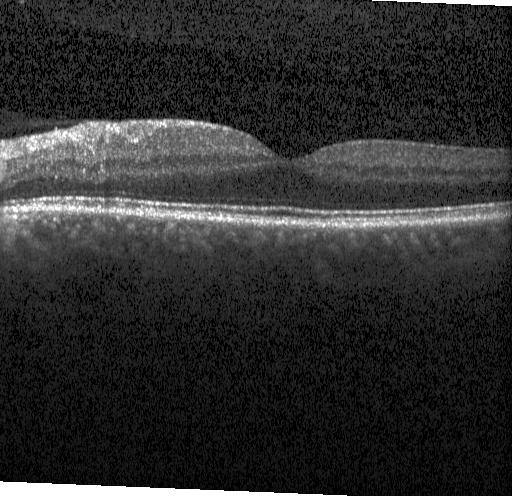 Diagnosis: neither choroidal neovascularization, diabetic macular edema, nor drusen.